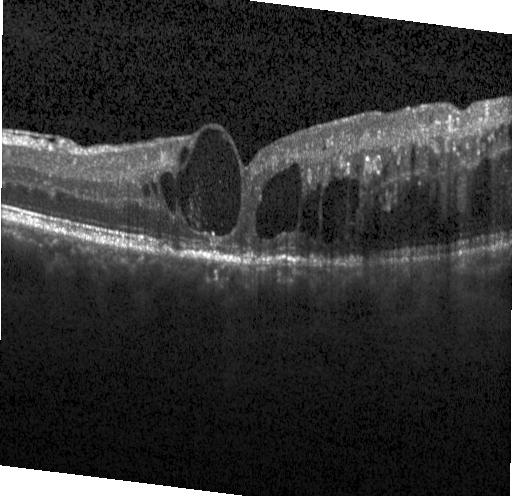

SD-OCT. Optical coherence tomography B-scan
This B-scan demonstrates DME.